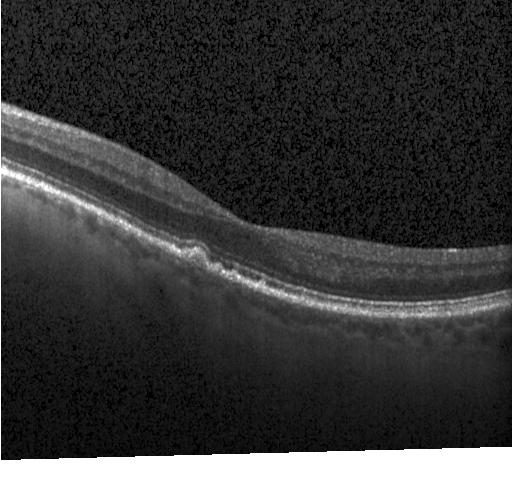
Optical coherence tomography B-scan. Sub-RPE drusenoid deposits.